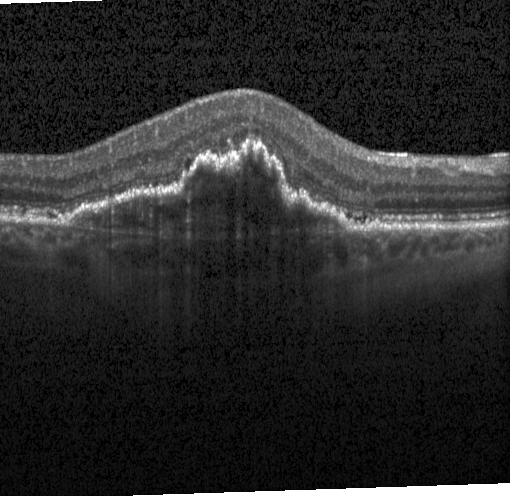 Diagnosis: a choroidal neovascular membrane.